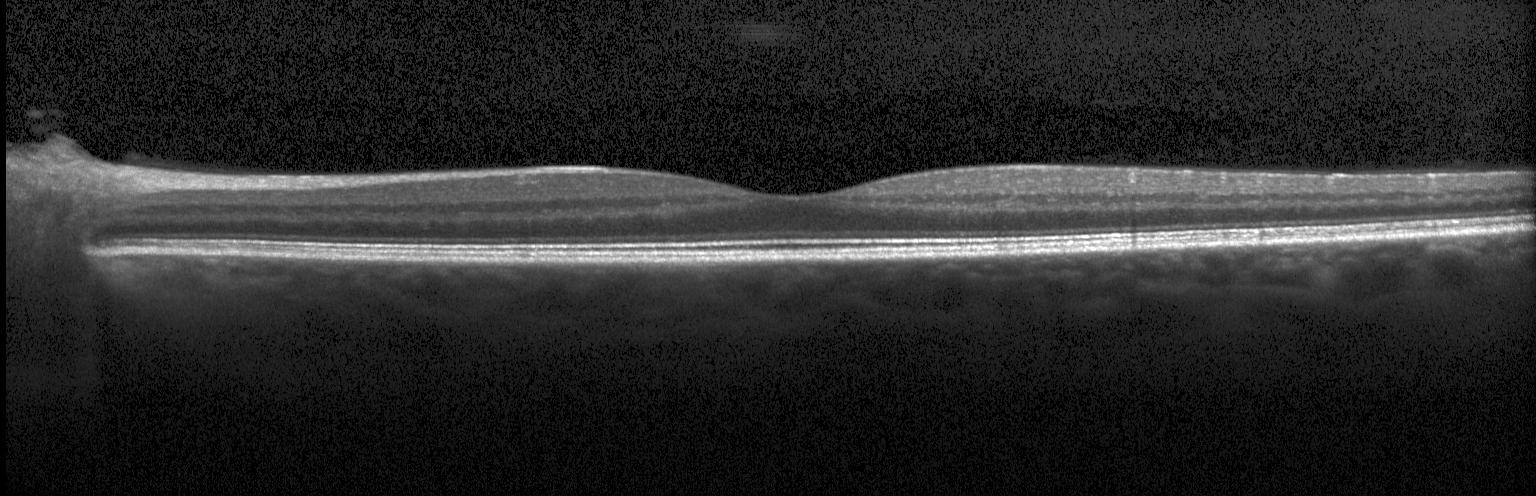

Horizontal scan through the fovea; retinal OCT B-scan; Heidelberg Spectralis OCT system
Finding: no CNV, no DME, and no drusen.